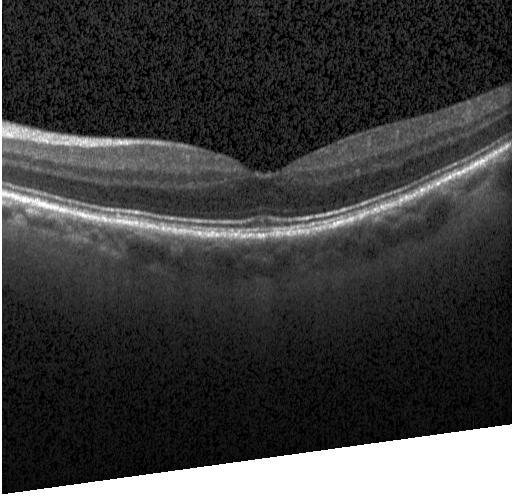

Centered on the fovea · instrument: Heidelberg Spectralis · OCT B-scan. Assessment: no evidence of CNV, DME, or drusen.